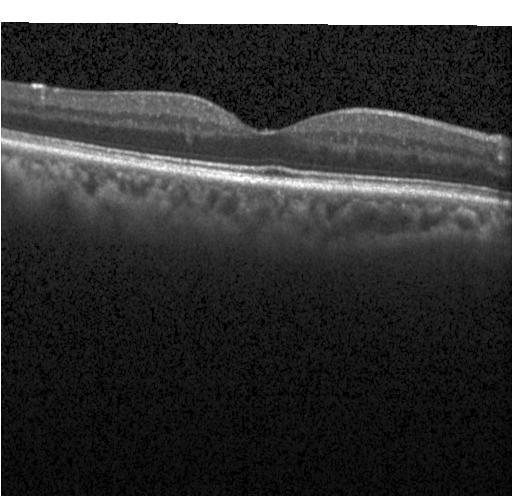 Optical coherence tomography B-scan. OCT finding: no choroidal neovascularization, no diabetic macular edema, and no drusen.